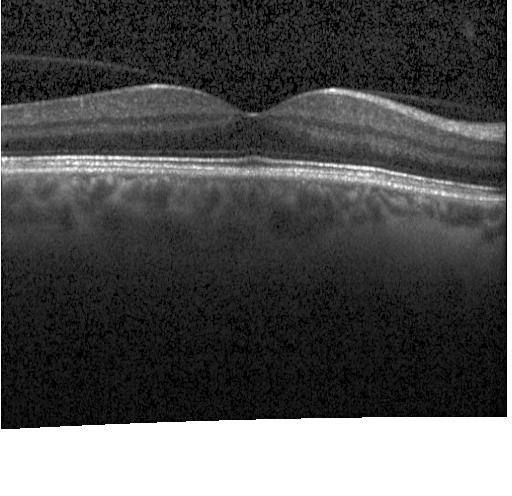 Heidelberg Spectralis · retinal OCT cross-section. Assessment: no choroidal neovascularization, no diabetic macular edema, and no drusen.